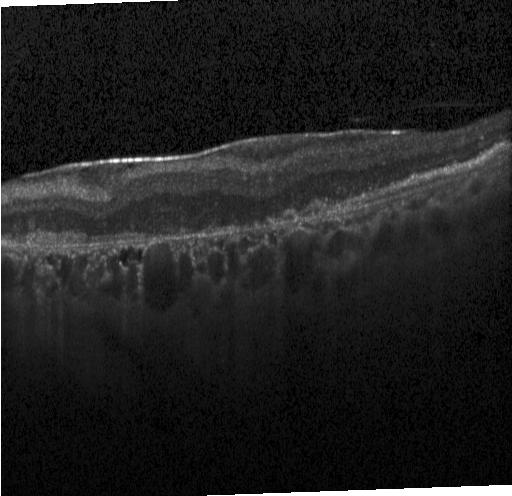

Retinal OCT cross-section · through the macula · acquired on a Heidelberg Spectralis · SD-OCT — A choroidal neovascular membrane.